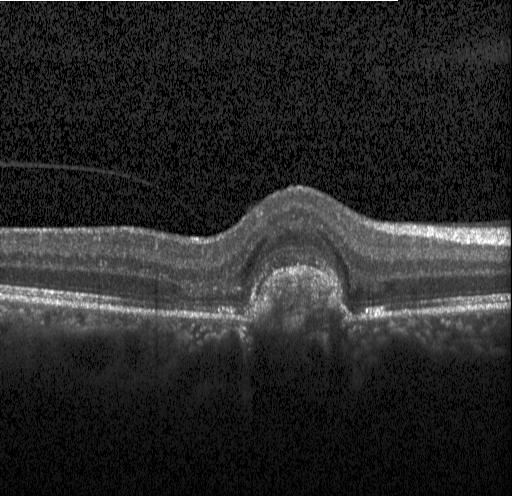
Centered on the fovea · Heidelberg Spectralis · retinal OCT B-scan — Impression: a choroidal neovascular membrane.